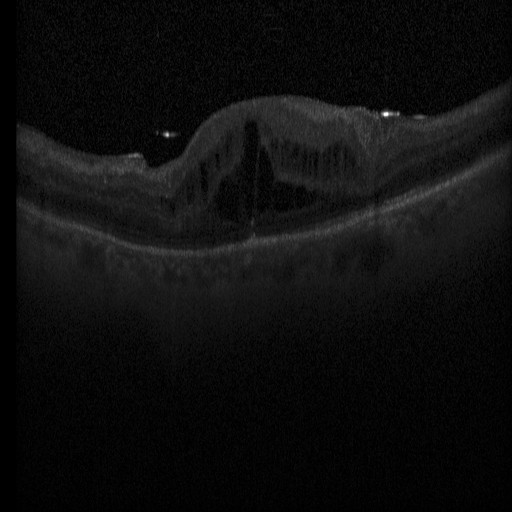
Retinal OCT cross-section
DME.